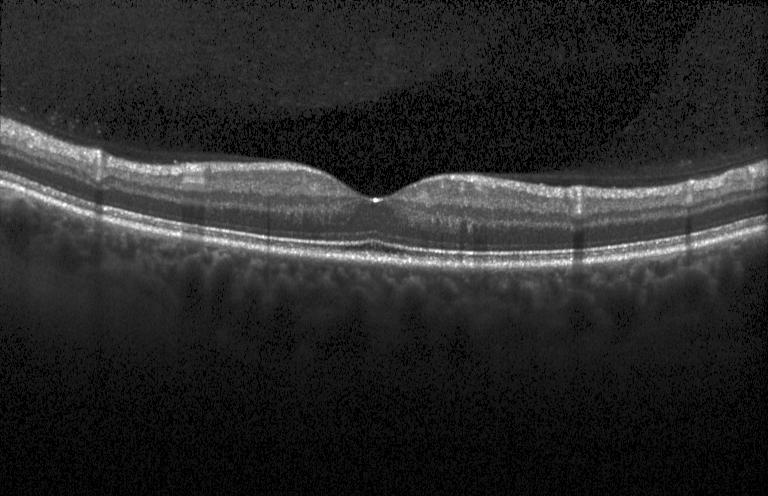
OCT B-scan. Spectral-domain optical coherence tomography — Finding: no choroidal neovascularization, no diabetic macular edema, and no drusen.